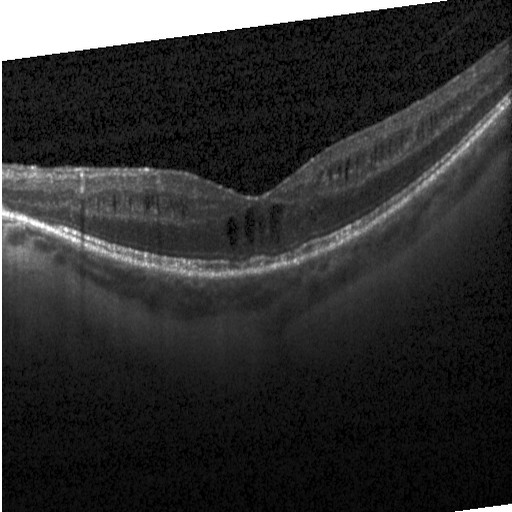
Spectral-domain OCT · optical coherence tomography scan · Heidelberg Spectralis · fovea-centered.
Diagnosis: diabetic macular edema.